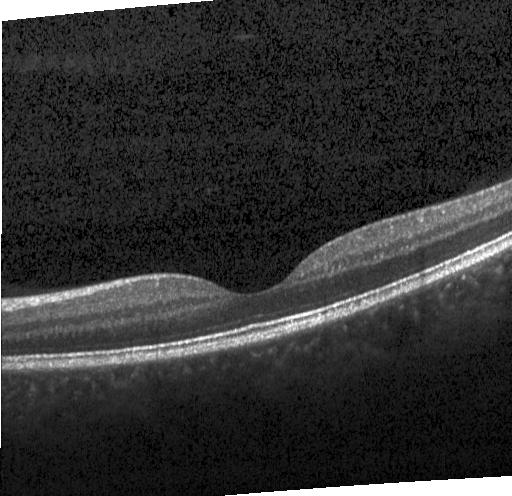 Spectral-domain optical coherence tomography, centered on the fovea, retinal OCT B-scan
The scan shows neither choroidal neovascularization, diabetic macular edema, nor drusen.